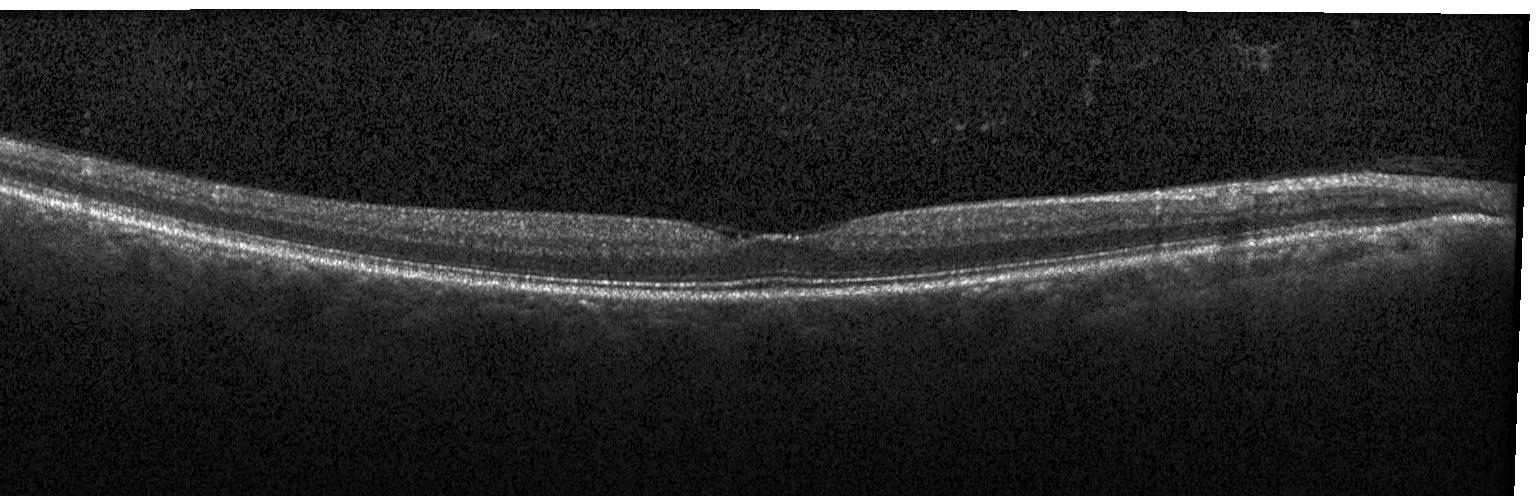
Optical coherence tomography scan. This B-scan demonstrates no evidence of choroidal neovascularization, diabetic macular edema, or drusen.